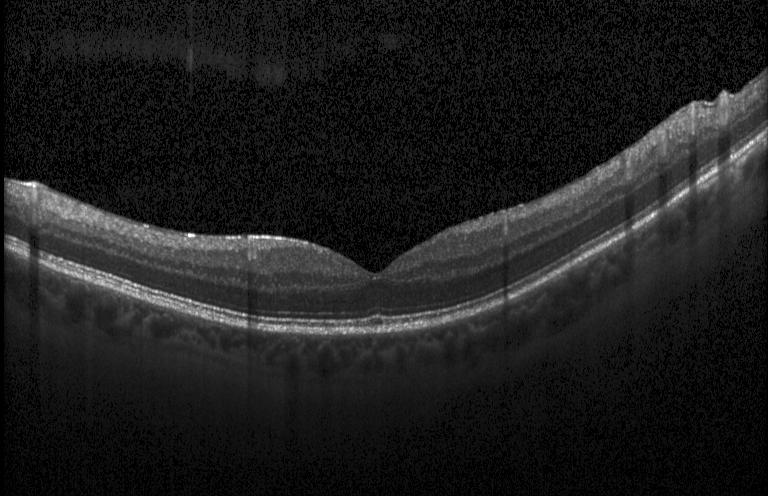 OCT finding: no evidence of choroidal neovascularization, diabetic macular edema, or drusen.